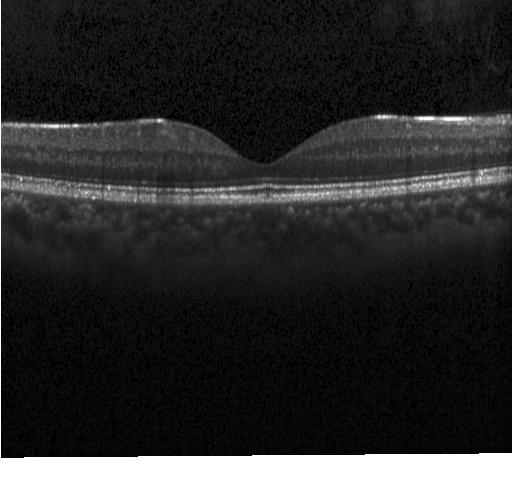 Spectral-domain optical coherence tomography · centered on the fovea · retinal OCT cross-section · Heidelberg Spectralis OCT system
Diagnosis: neither choroidal neovascularization, diabetic macular edema, nor drusen.